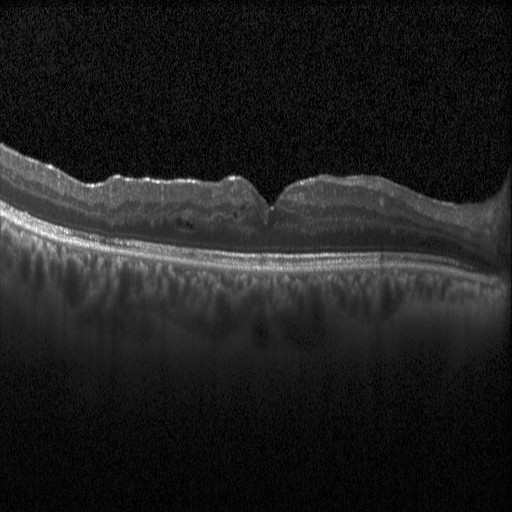 Horizontal scan through the fovea, retinal OCT B-scan
Diabetic macular edema.